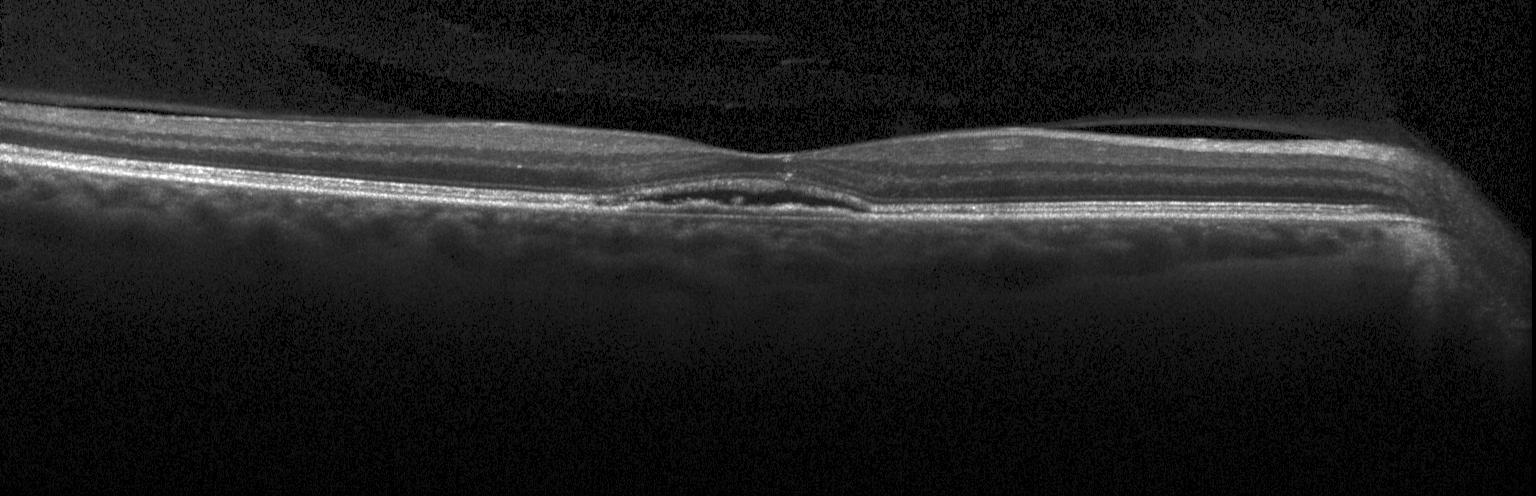 Dx: choroidal neovascularization.